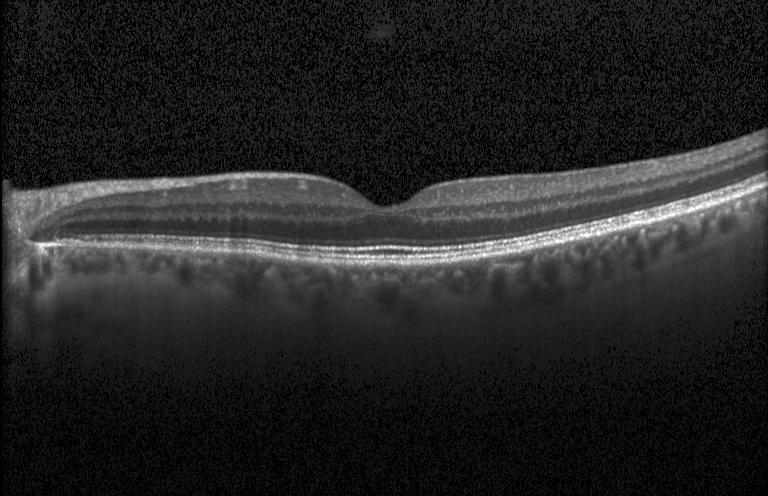

Spectral-domain optical coherence tomography, OCT line scan, through the macula
Impression: no evidence of CNV, DME, or drusen.